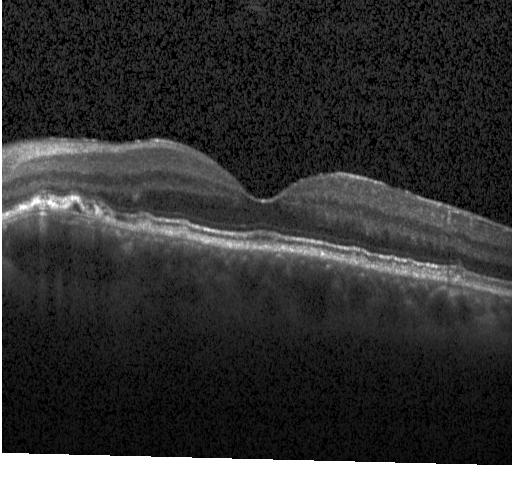

Diagnosis: sub-RPE drusenoid deposits.